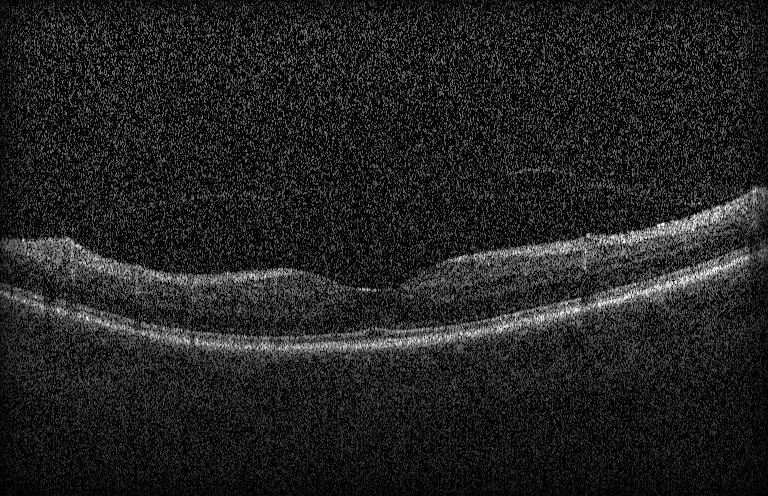
Retinal OCT cross-section · spectral-domain optical coherence tomography. Diagnosis: neither choroidal neovascularization, diabetic macular edema, nor drusen.